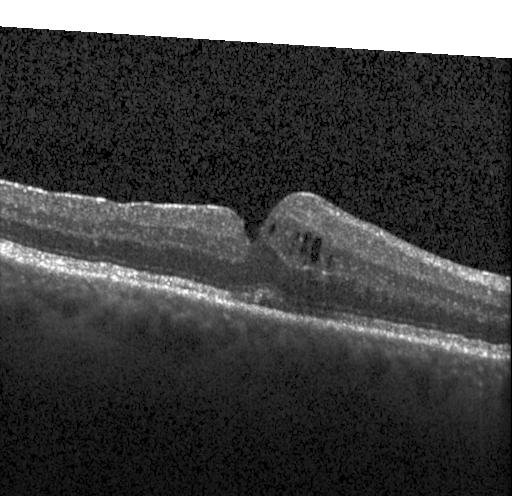 OCT B-scan — Impression: diabetic macular edema (DME).